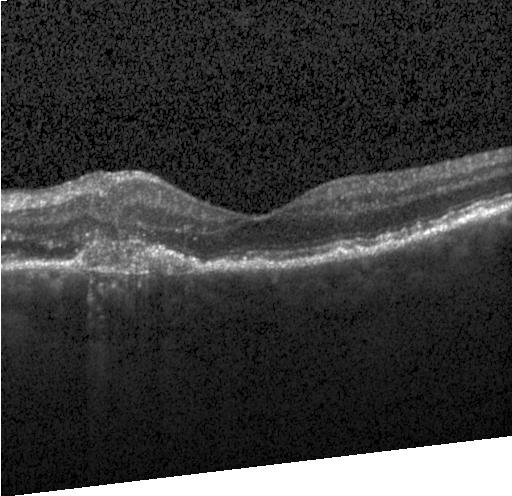
Retinal OCT B-scan
Dx: a choroidal neovascular membrane.